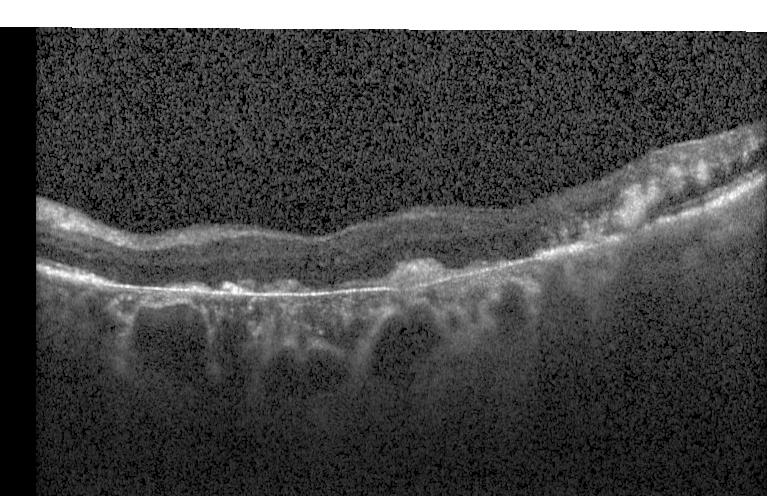

Instrument: Heidelberg Spectralis; OCT line scan — Finding: a choroidal neovascular membrane.